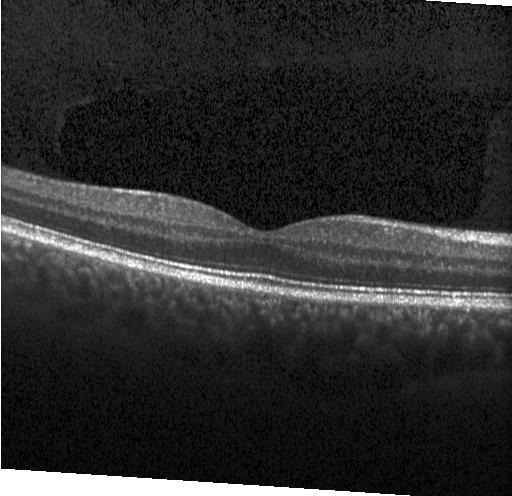

Finding: no choroidal neovascularization, diabetic macular edema, or drusen.